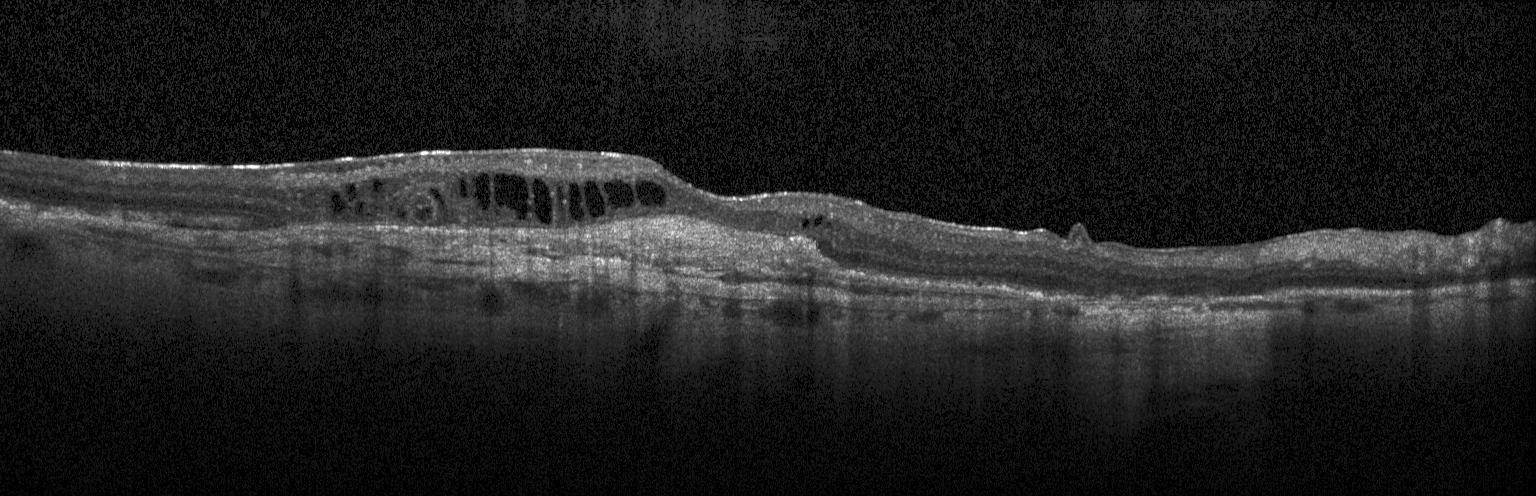
Horizontal scan through the fovea, spectral-domain optical coherence tomography, retinal OCT cross-section
Impression: a choroidal neovascular membrane.